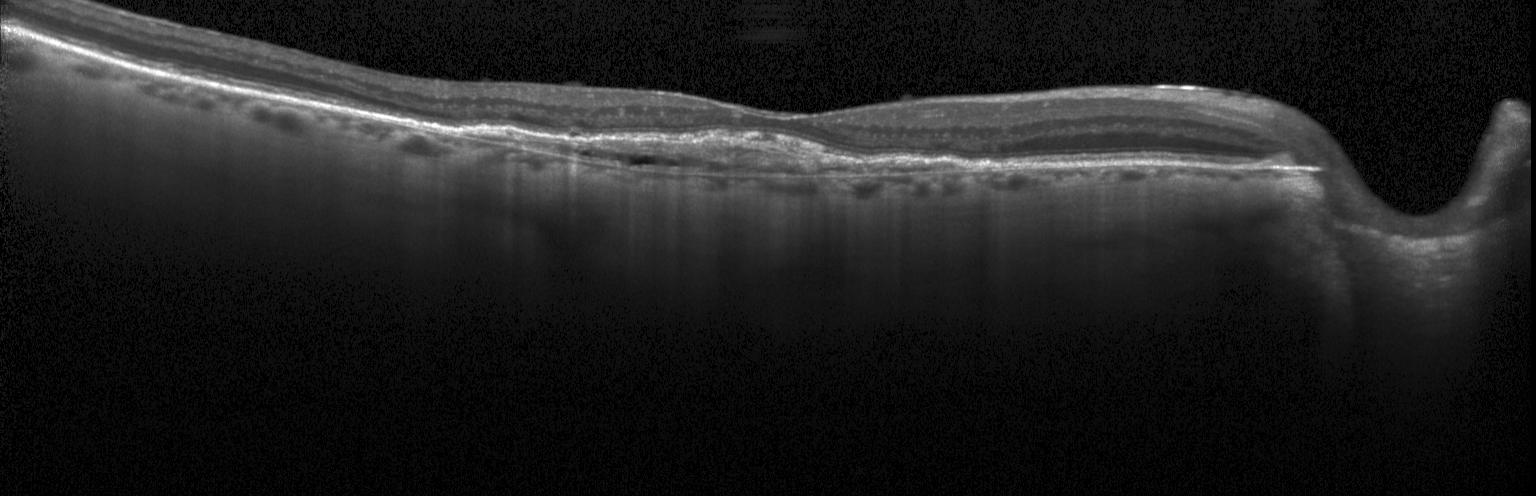 Impression: a choroidal neovascular membrane.